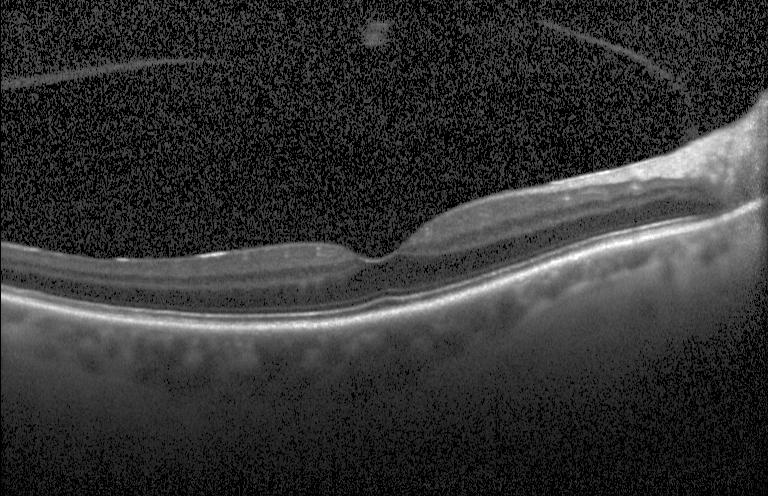

Spectral-domain OCT · retinal OCT B-scan · Heidelberg Spectralis · fovea-centered
OCT finding: no choroidal neovascularization, no diabetic macular edema, and no drusen.